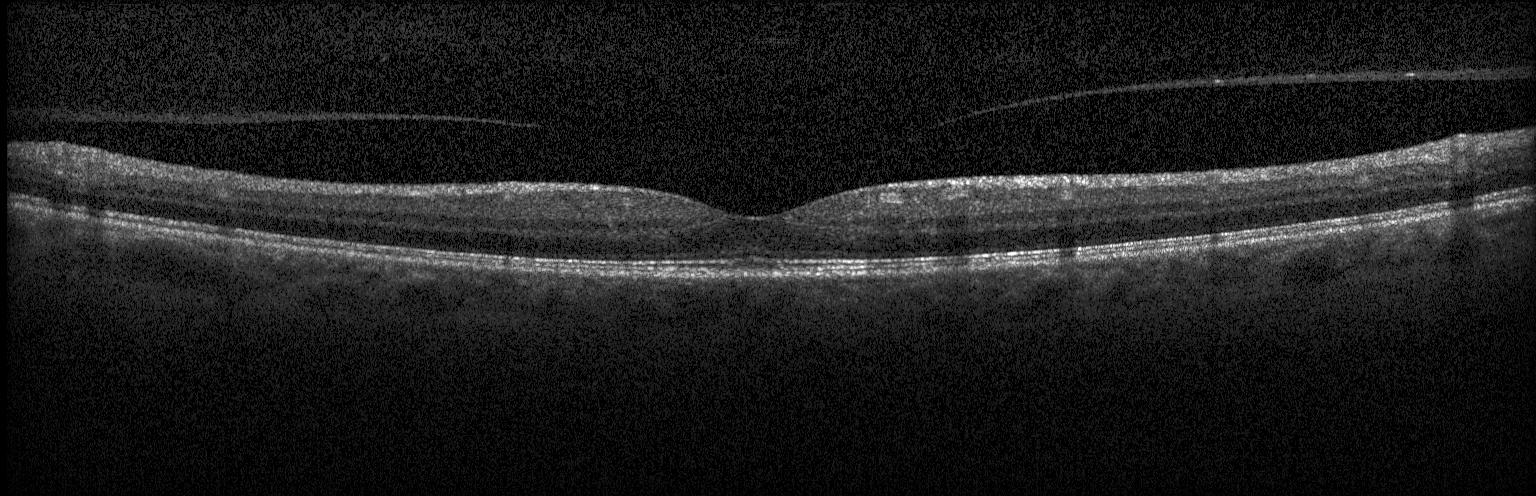
Macular scan. OCT line scan. Heidelberg Spectralis OCT system. Spectral-domain OCT
Impression: no choroidal neovascularization, no diabetic macular edema, and no drusen.